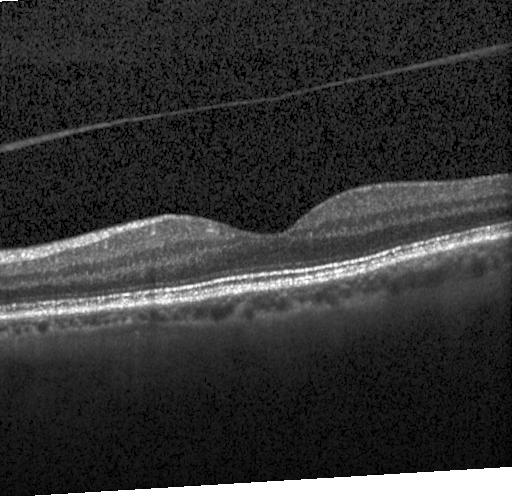
Retinal OCT cross-section
OCT finding: no CNV, DME, or drusen.